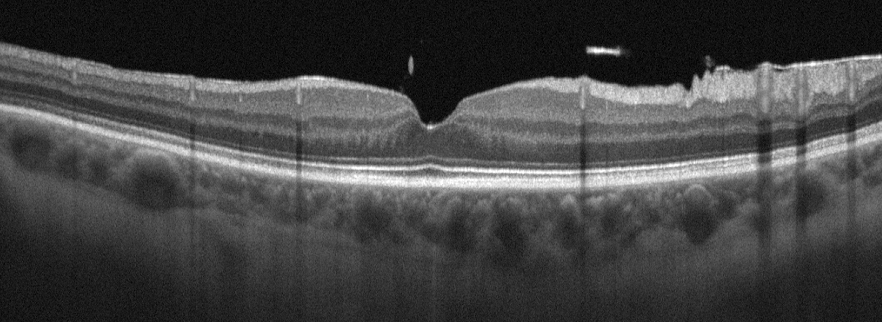 Optovue Avanti RTVue XR · macular scan · retinal OCT cross-section
Finding: epiretinal membrane (ERM).